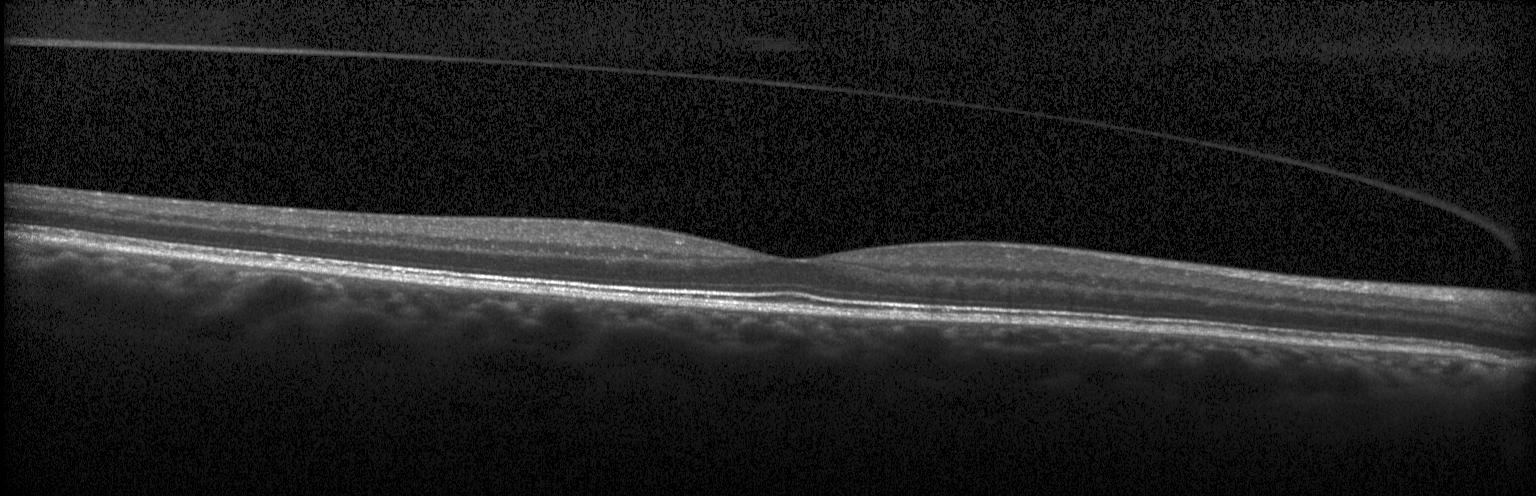 SD-OCT. Optical coherence tomography scan
This B-scan demonstrates no evidence of choroidal neovascularization, diabetic macular edema, or drusen.